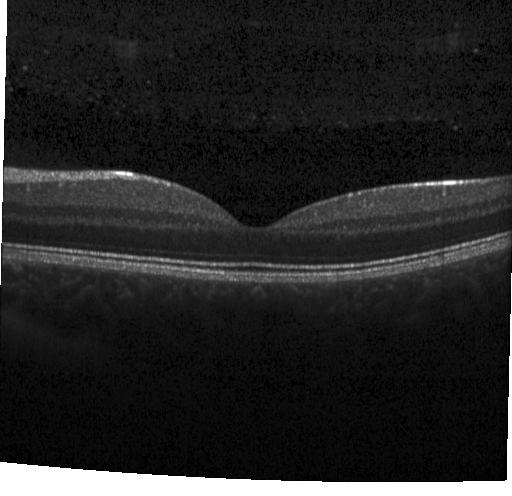 Retinal OCT B-scan. Diagnosis: no choroidal neovascularization, diabetic macular edema, or drusen.